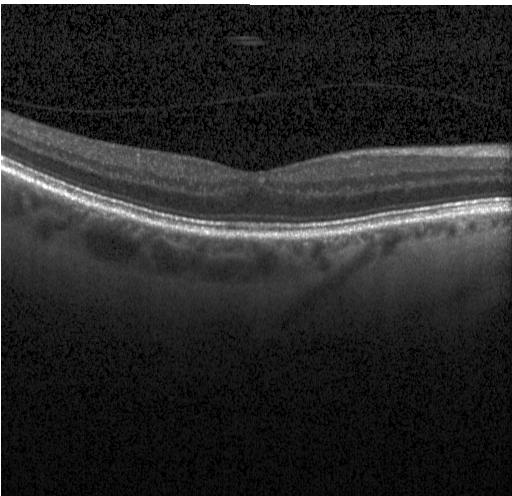 OCT finding: no choroidal neovascularization, no diabetic macular edema, and no drusen.